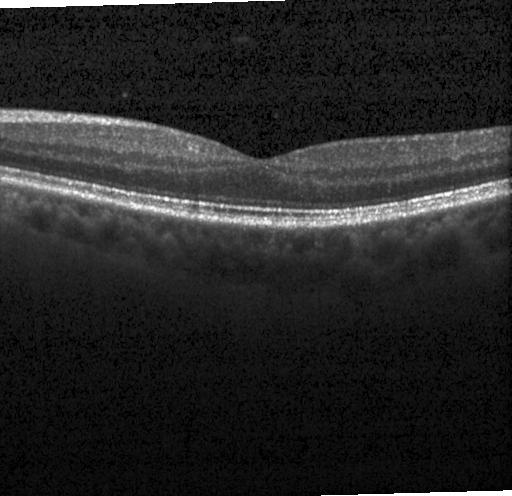 Retinal OCT B-scan, macular scan, spectral-domain optical coherence tomography
Macular OCT: no choroidal neovascularization, diabetic macular edema, or drusen.